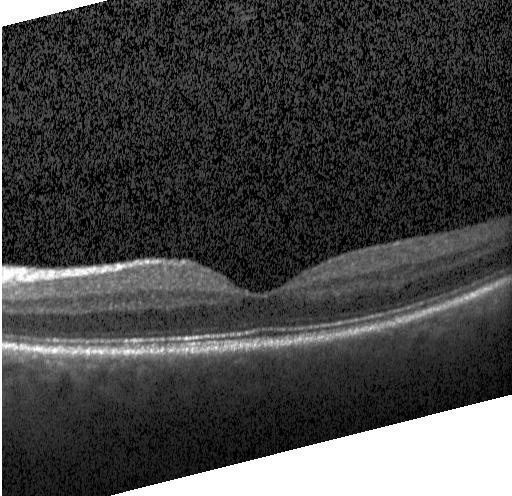 Macular scan · acquired on a Heidelberg Spectralis · retinal OCT cross-section — Finding: neither choroidal neovascularization, diabetic macular edema, nor drusen.